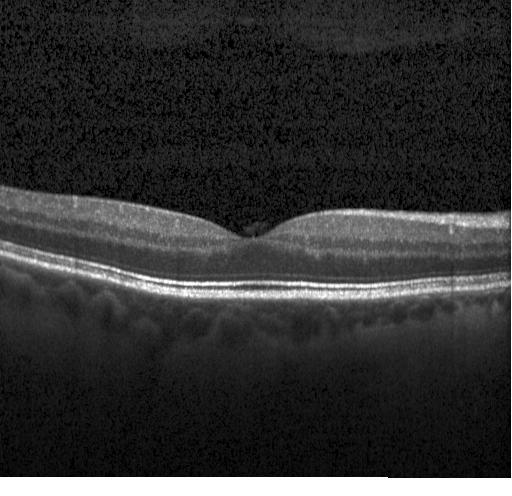

Finding: no choroidal neovascularization, diabetic macular edema, or drusen.